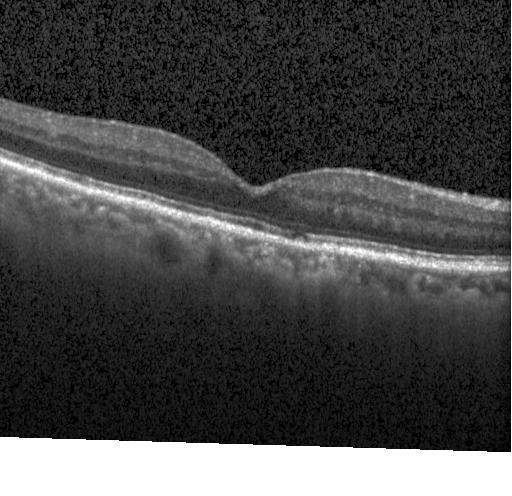 Instrument: Heidelberg Spectralis. Horizontal scan through the fovea. Retinal OCT cross-section
The scan shows neither choroidal neovascularization, diabetic macular edema, nor drusen.